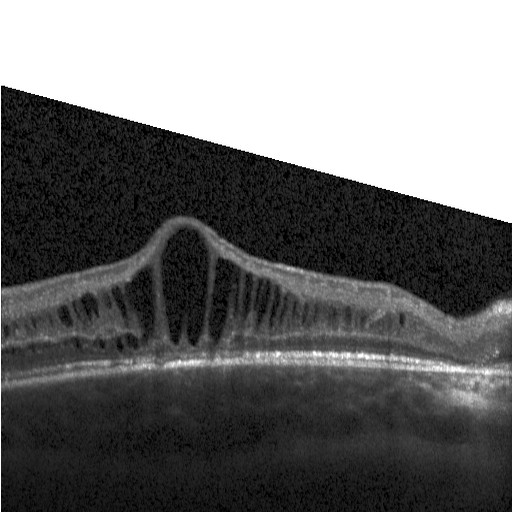
Retinal OCT B-scan
Macular OCT: diabetic macular edema (DME).